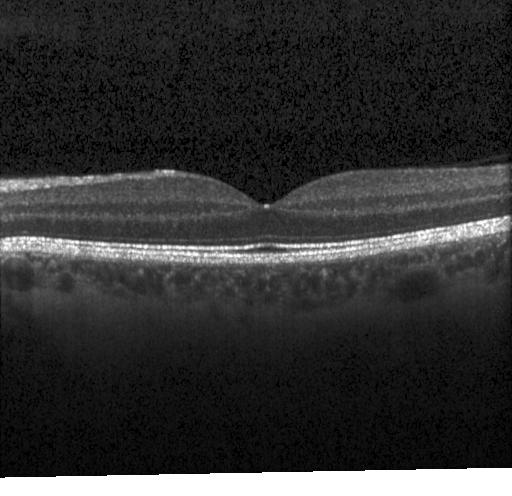
This B-scan demonstrates no evidence of choroidal neovascularization, diabetic macular edema, or drusen.